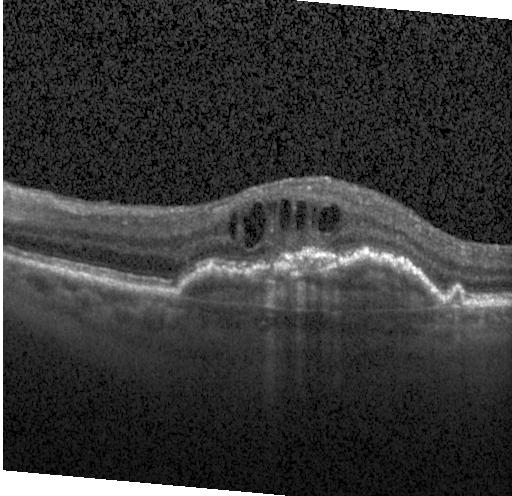 Finding: CNV.